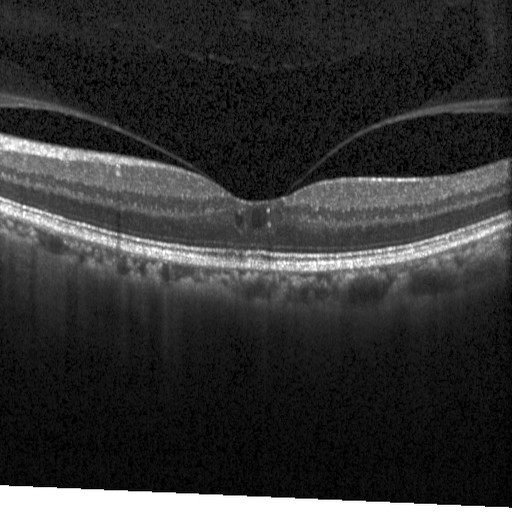

Spectral-domain OCT. Optical coherence tomography scan
DME.